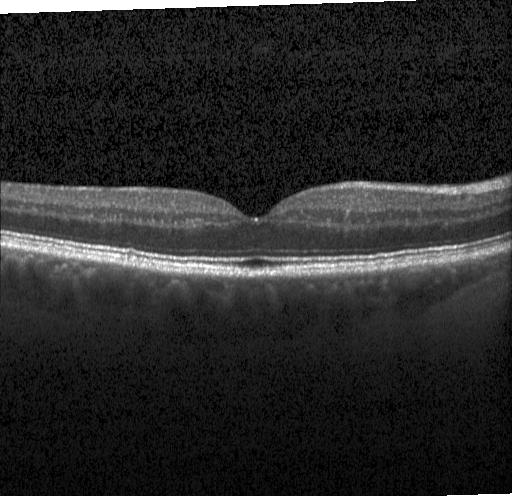
Diagnosis: no evidence of choroidal neovascularization, diabetic macular edema, or drusen.